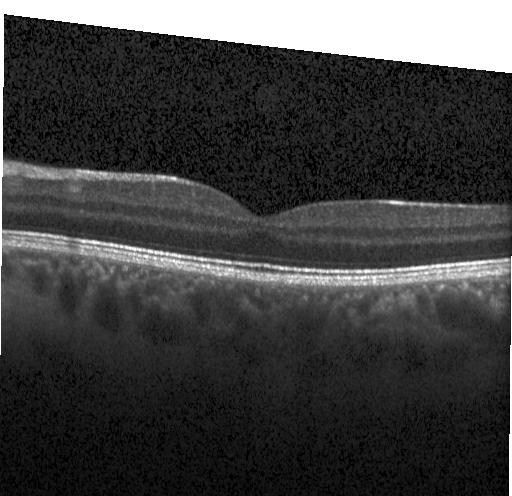

Acquired on a Heidelberg Spectralis; optical coherence tomography scan; SD-OCT; horizontal scan through the fovea — This B-scan demonstrates no choroidal neovascularization, no diabetic macular edema, and no drusen.